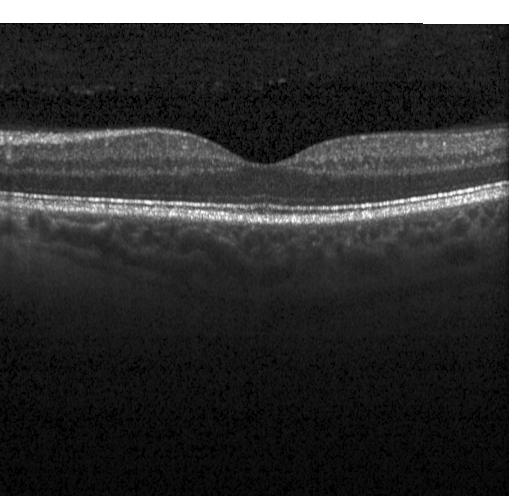
Impression: no choroidal neovascularization, diabetic macular edema, or drusen.